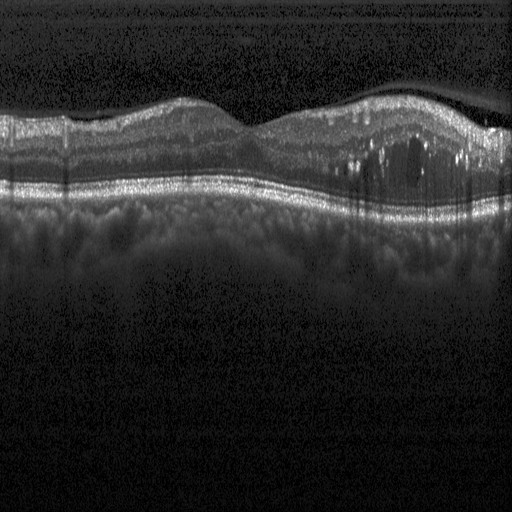

OCT B-scan — Diagnosis: DME.